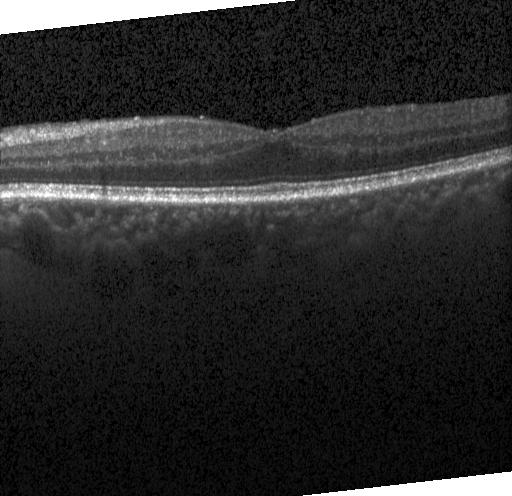
Retinal OCT cross-section showing no evidence of choroidal neovascularization, diabetic macular edema, or drusen.